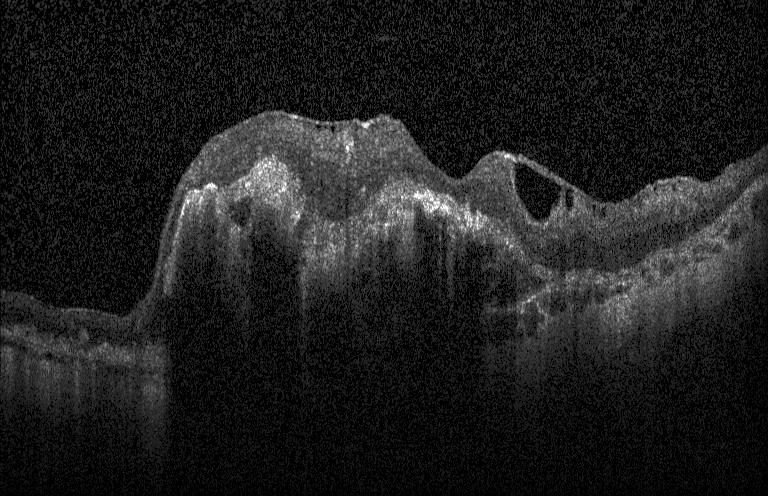
Optical coherence tomography scan; horizontal scan through the fovea.
Diagnosis: choroidal neovascularization (CNV).